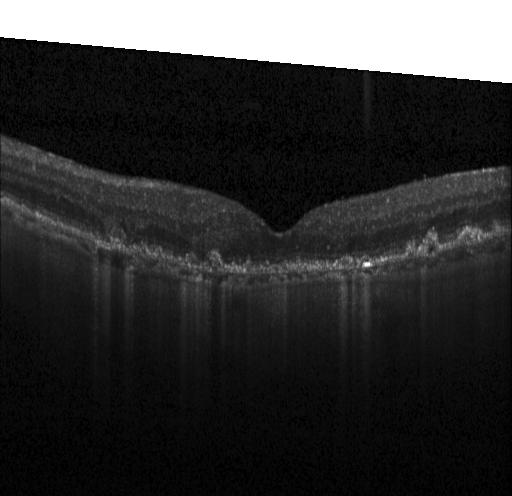 OCT scan showing a choroidal neovascular membrane.